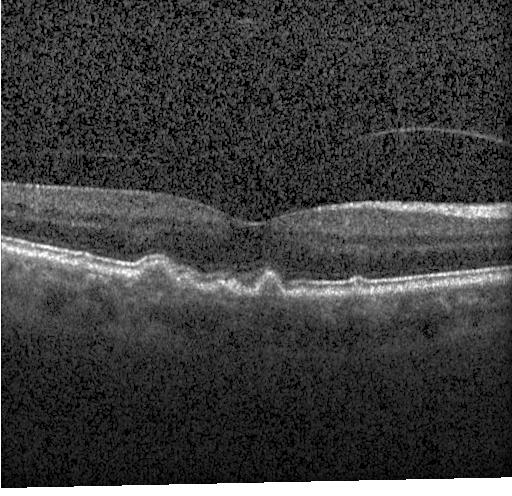 OCT B-scan · Heidelberg Spectralis OCT system.
The scan shows sub-RPE drusenoid deposits.